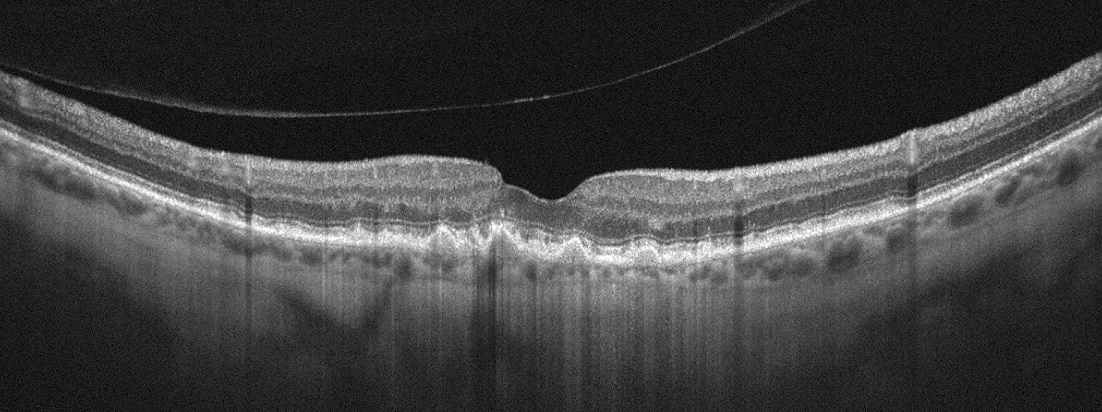
Optical coherence tomography scan, acquired on an Optovue Avanti RTVue XR, fovea-centered.
Dx: age-related macular degeneration (AMD).